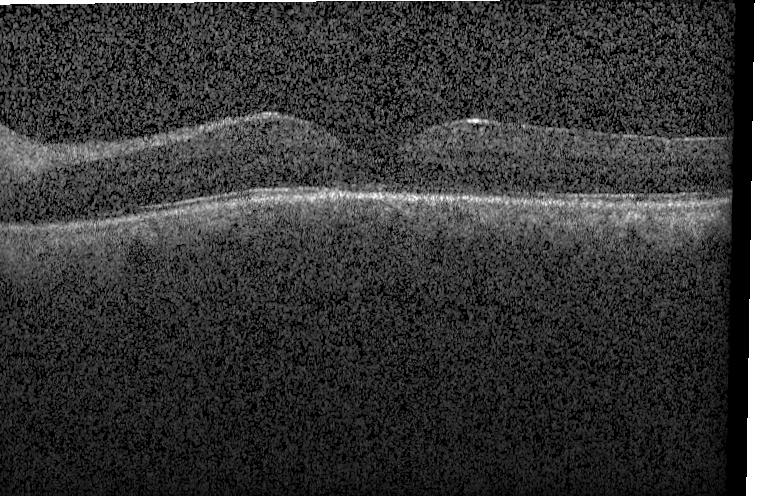 Retinal OCT cross-section — Assessment: neither choroidal neovascularization, diabetic macular edema, nor drusen.